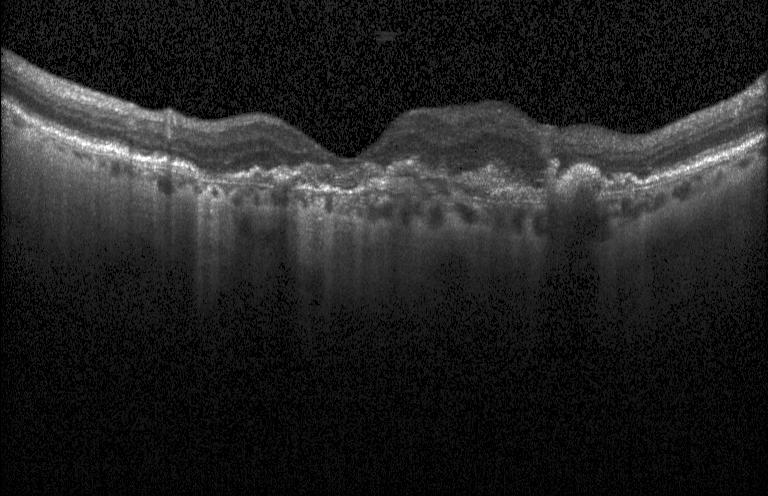

Retinal OCT cross-section.
OCT finding: CNV.